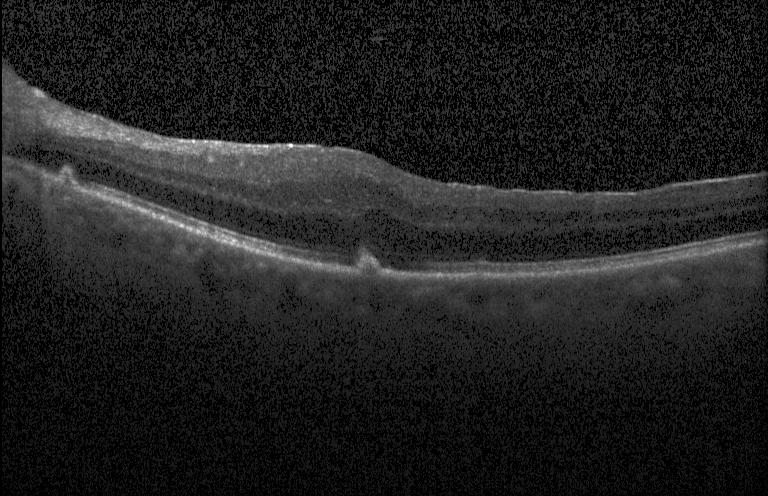

Multiple drusen.